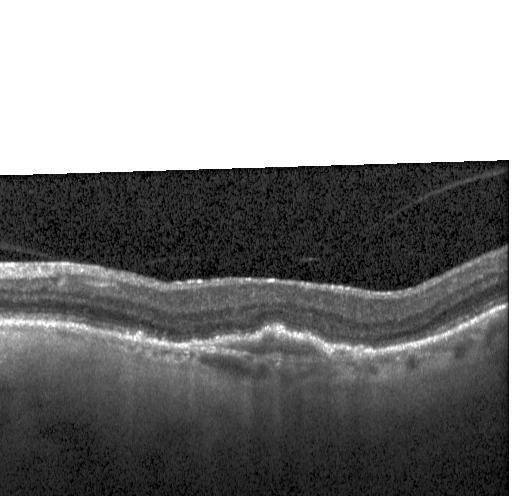 Retinal OCT cross-section — Finding: choroidal neovascularization (CNV).